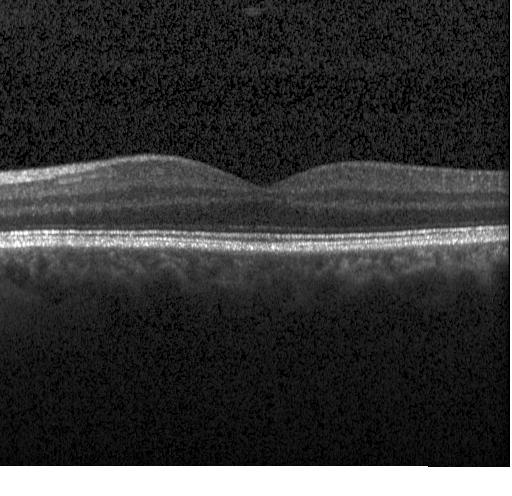 Impression: neither choroidal neovascularization, diabetic macular edema, nor drusen.